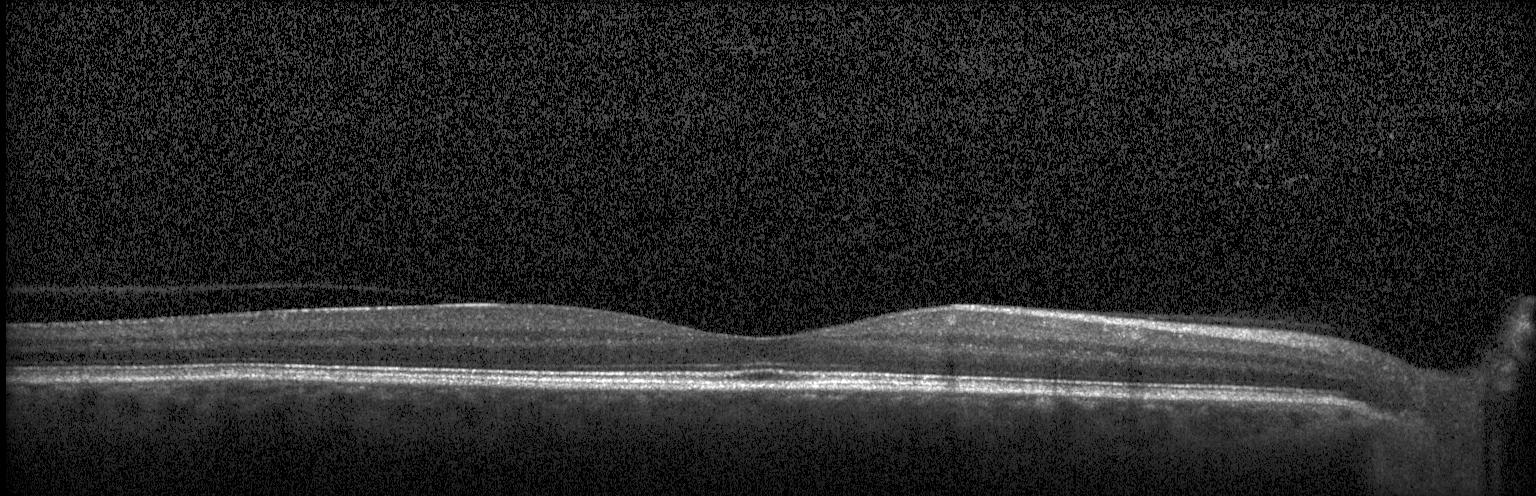 Spectral-domain OCT. Fovea-centered. OCT B-scan.
This B-scan demonstrates neither choroidal neovascularization, diabetic macular edema, nor drusen.